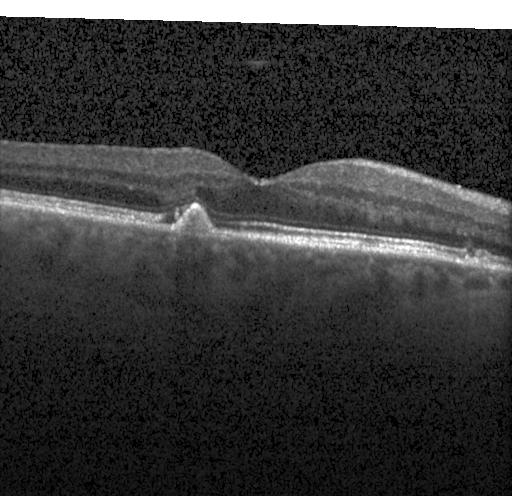

This B-scan demonstrates choroidal neovascularization (CNV).